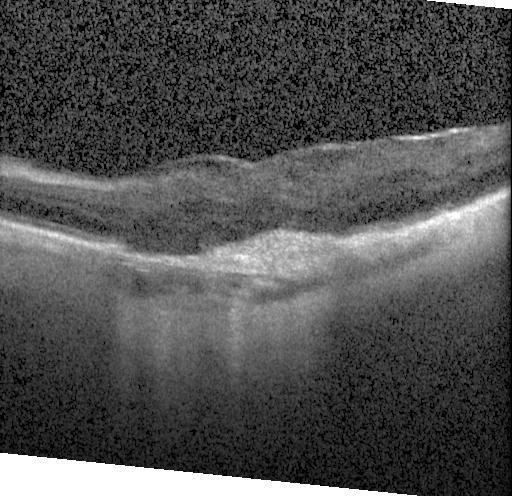

OCT B-scan
A choroidal neovascular membrane.